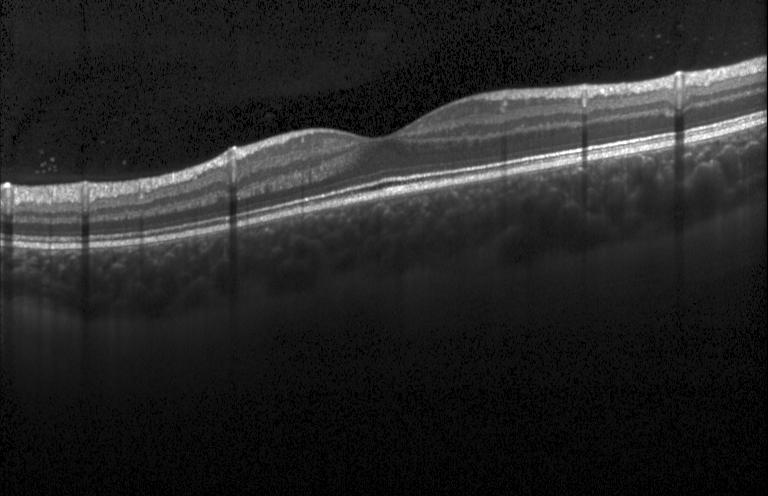
Spectral-domain OCT B-scan: no choroidal neovascularization, diabetic macular edema, or drusen.